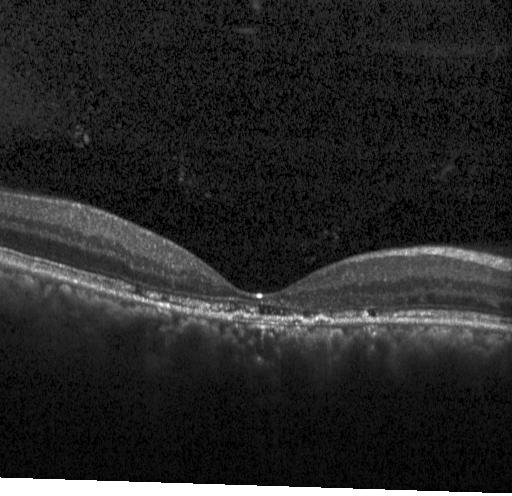

Finding: CNV.